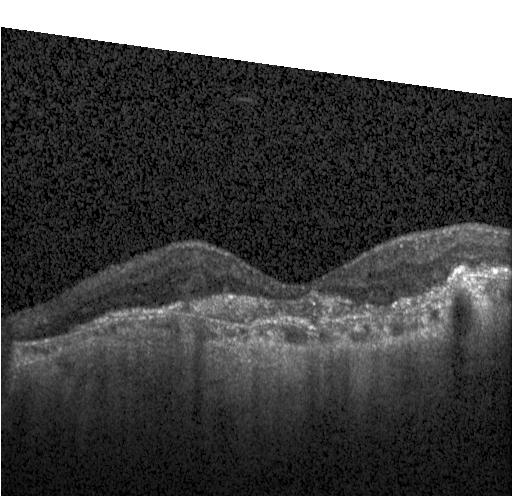

OCT scan showing CNV.